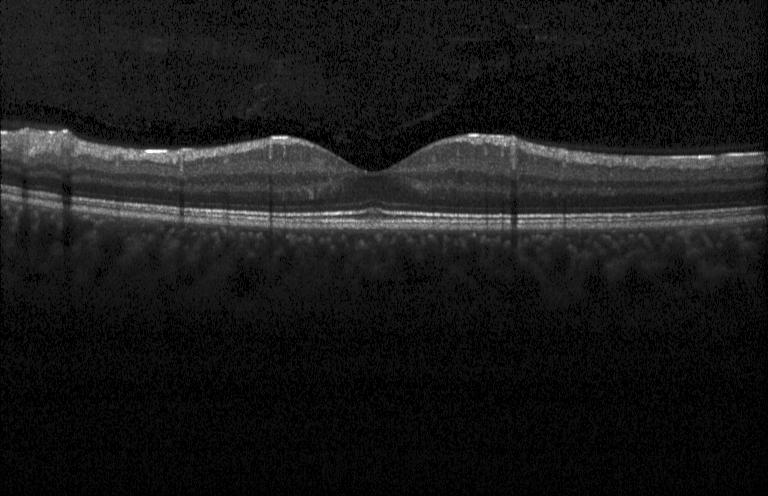
Impression: no CNV, DME, or drusen.